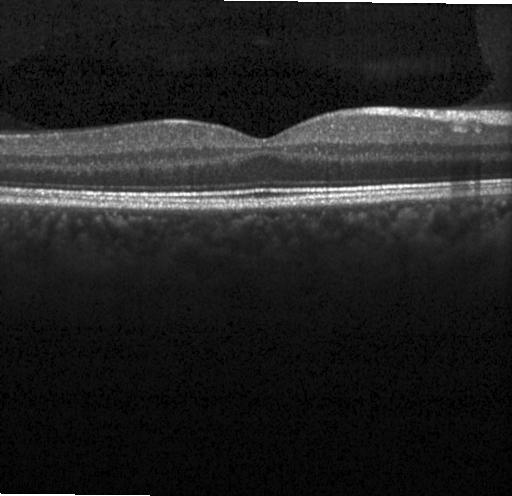

OCT line scan; acquired on a Heidelberg Spectralis. OCT finding: no choroidal neovascularization, no diabetic macular edema, and no drusen.